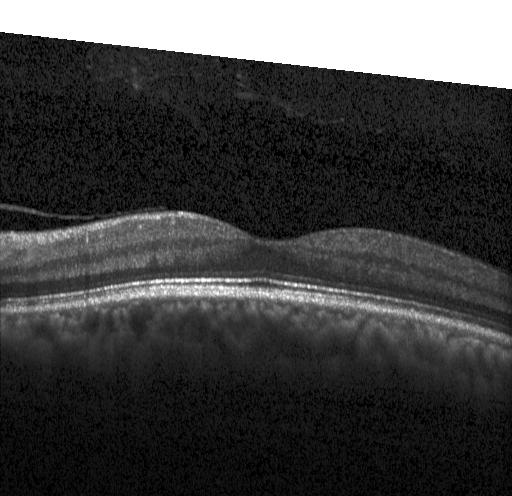
Impression: no choroidal neovascularization, no diabetic macular edema, and no drusen.